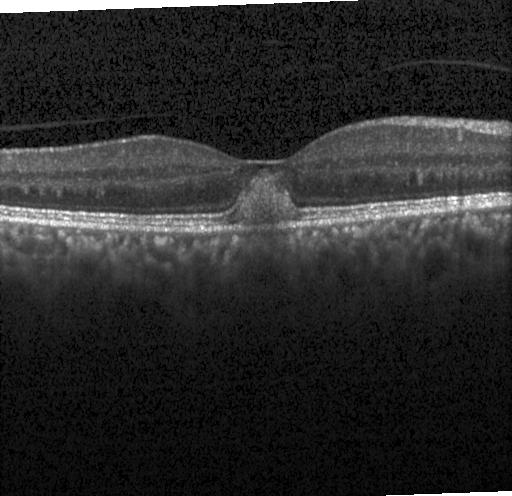
Through the macula, Heidelberg Spectralis, retinal OCT cross-section.
Dx: CNV.